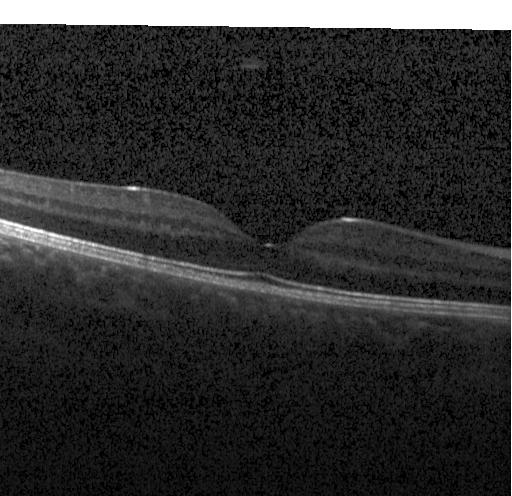

Retinal OCT cross-section. Finding: no choroidal neovascularization, diabetic macular edema, or drusen.